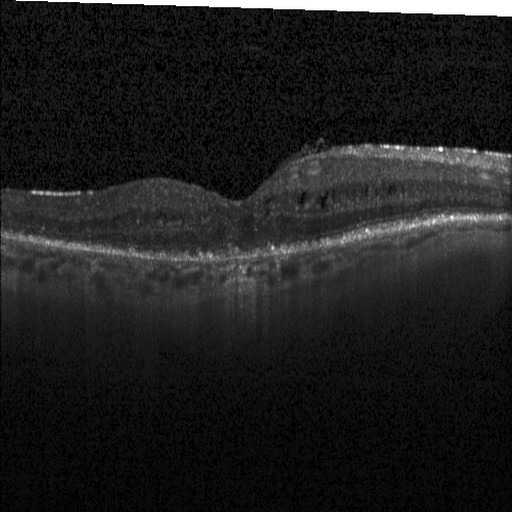
Optical coherence tomography scan, spectral-domain OCT, horizontal scan through the fovea
Assessment: diabetic macular edema (DME).